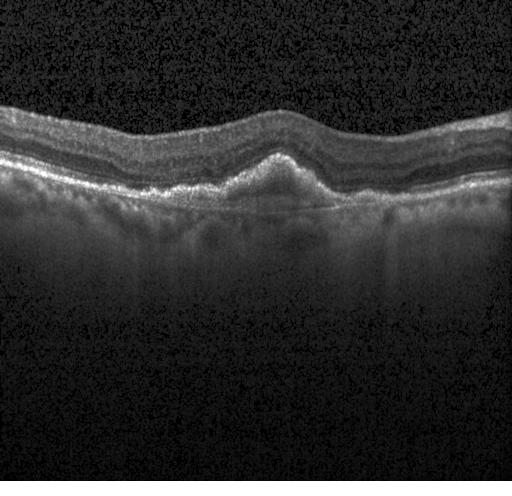
Spectral-domain optical coherence tomography, OCT line scan — Impression: choroidal neovascularization.